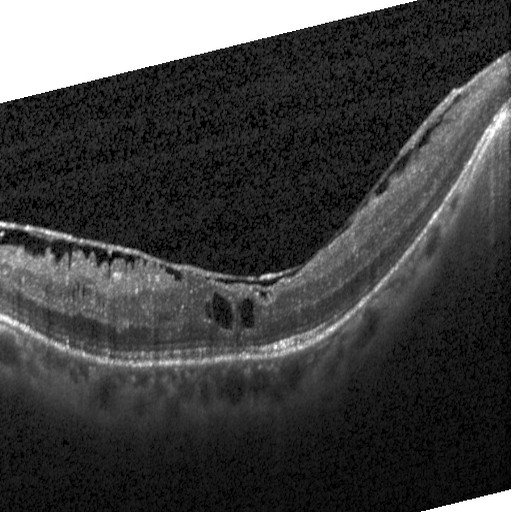
OCT finding: diabetic macular edema (DME).